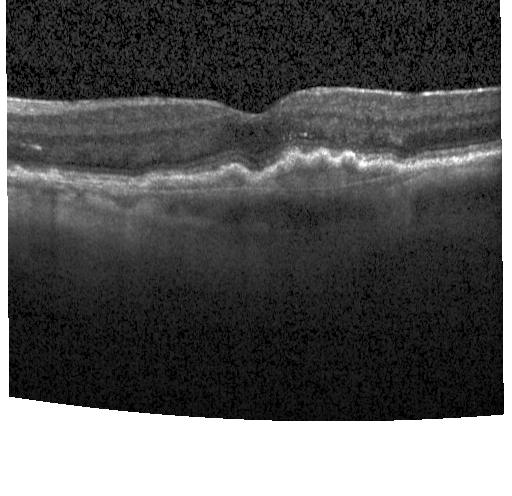
SD-OCT · through the macula · Heidelberg Spectralis OCT system · retinal OCT B-scan.
OCT finding: a choroidal neovascular membrane.